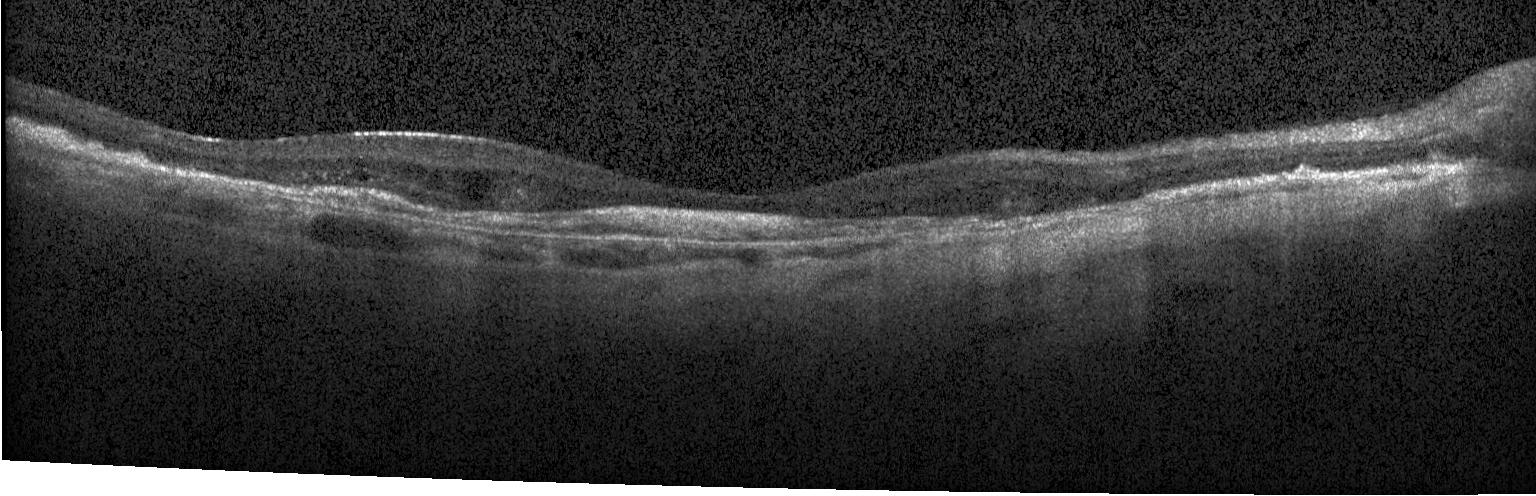

A choroidal neovascular membrane.